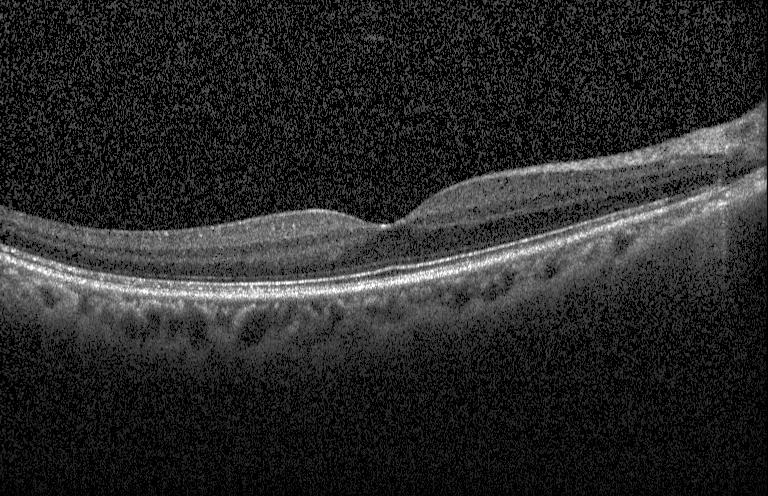 OCT line scan, spectral-domain optical coherence tomography. Diagnosis: no evidence of choroidal neovascularization, diabetic macular edema, or drusen.